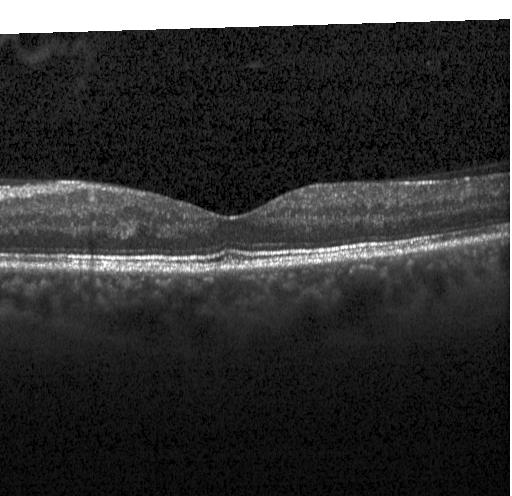
SD-OCT, retinal OCT B-scan.
OCT finding: no choroidal neovascularization, diabetic macular edema, or drusen.